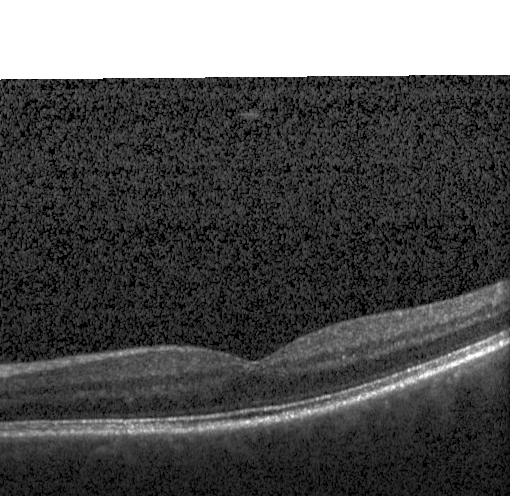
SD-OCT · OCT line scan · Heidelberg Spectralis OCT system · fovea-centered. Macular OCT: neither choroidal neovascularization, diabetic macular edema, nor drusen.